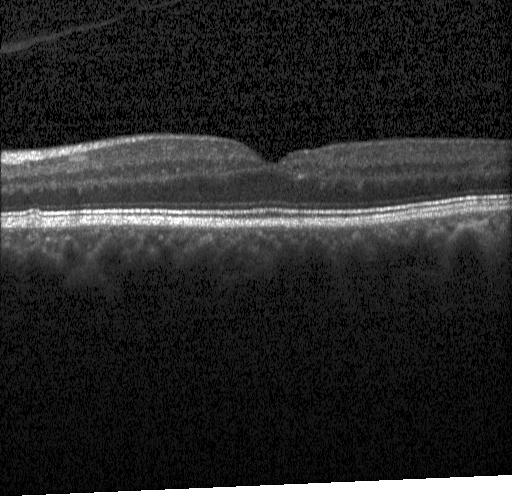

Finding: no CNV, no DME, and no drusen.